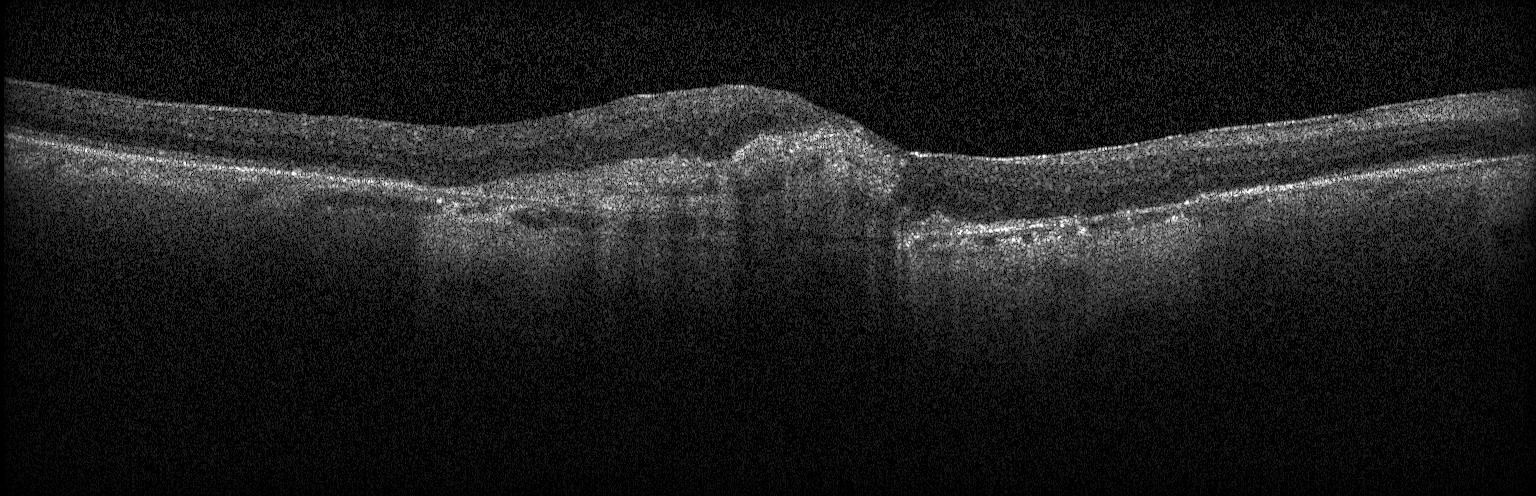
OCT scan showing CNV.